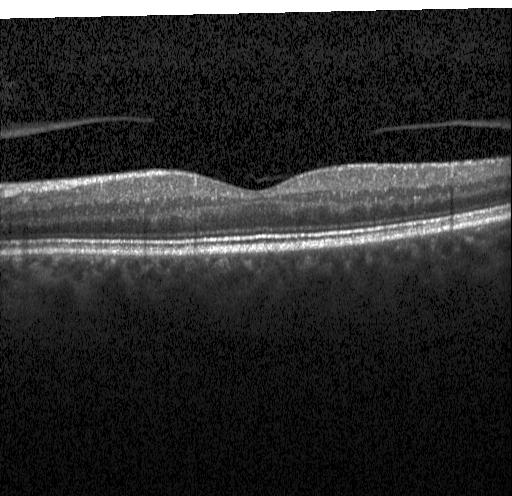
The scan shows no choroidal neovascularization, diabetic macular edema, or drusen.